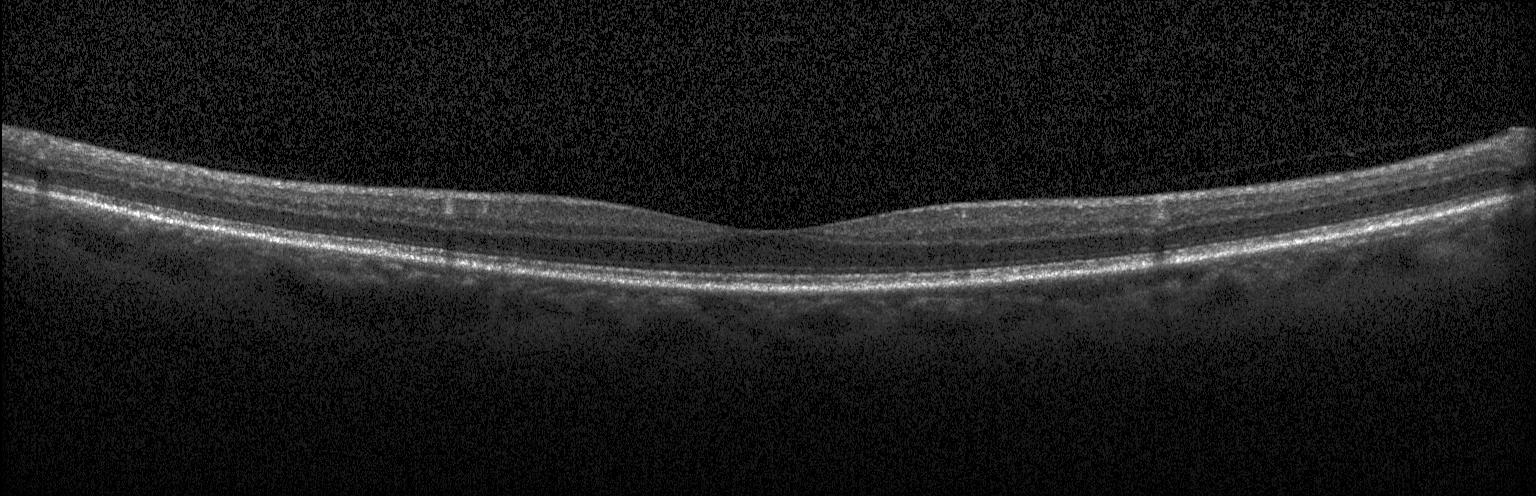
Acquired on a Heidelberg Spectralis · OCT B-scan
Diagnosis: neither CNV, DME, nor drusen.